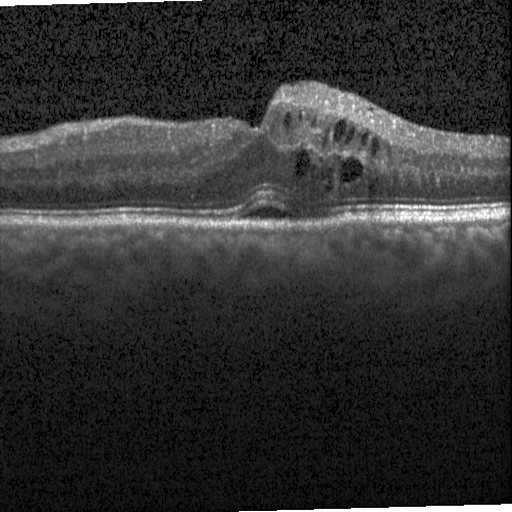 Retinal OCT cross-section.
Assessment: diabetic macular edema.